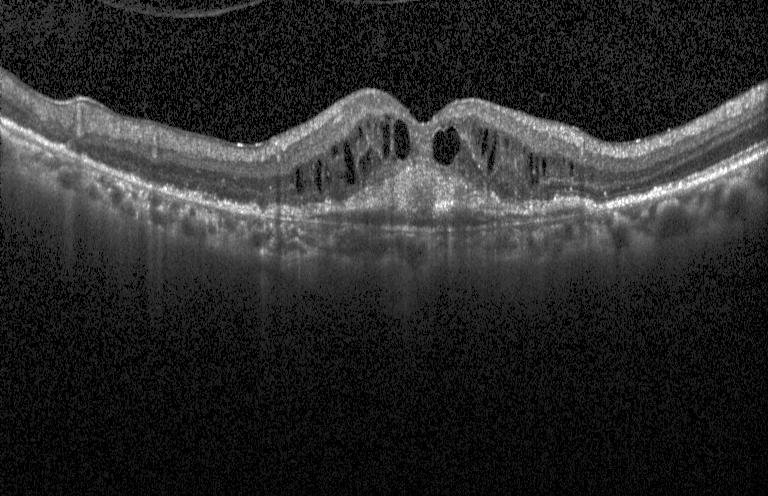
Dx: CNV.